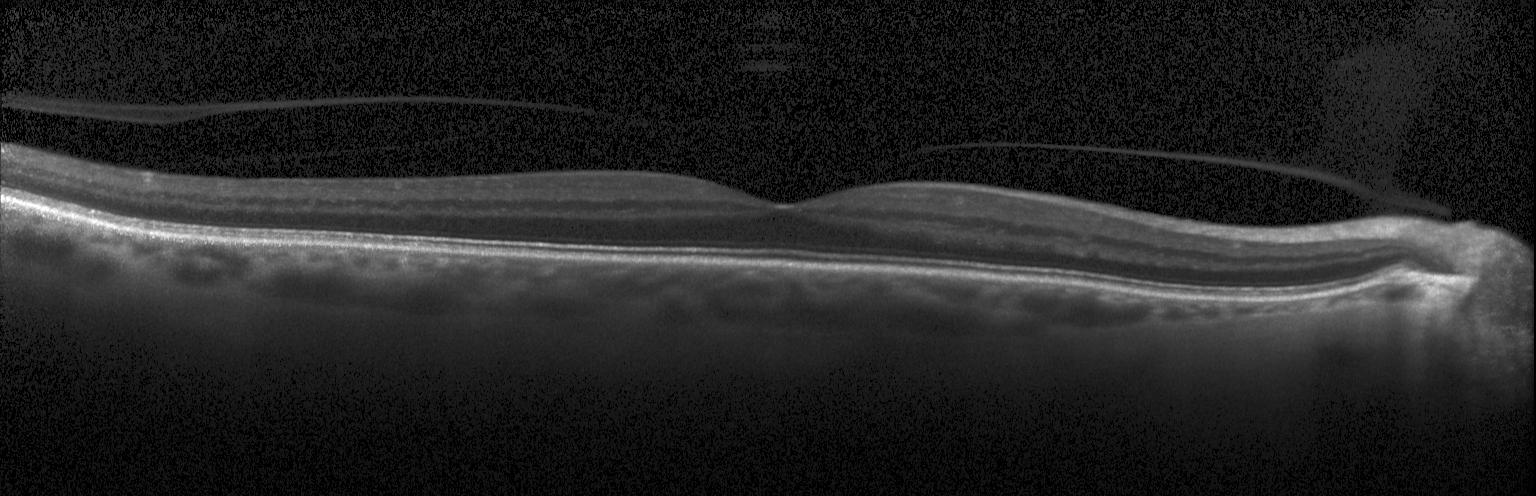
Spectral-domain OCT B-scan: no evidence of choroidal neovascularization, diabetic macular edema, or drusen.